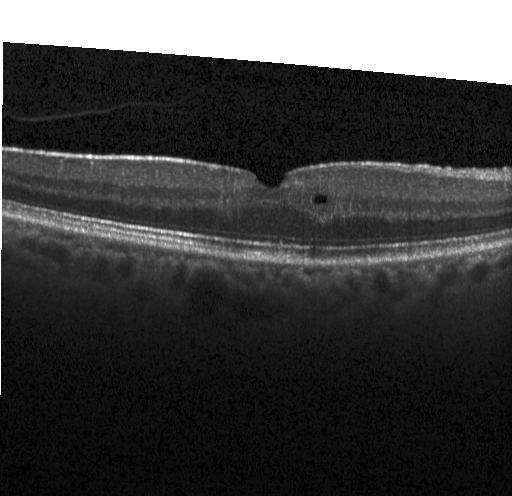
Acquired on a Heidelberg Spectralis; OCT line scan; macular scan; spectral-domain optical coherence tomography — OCT finding: diabetic macular edema.